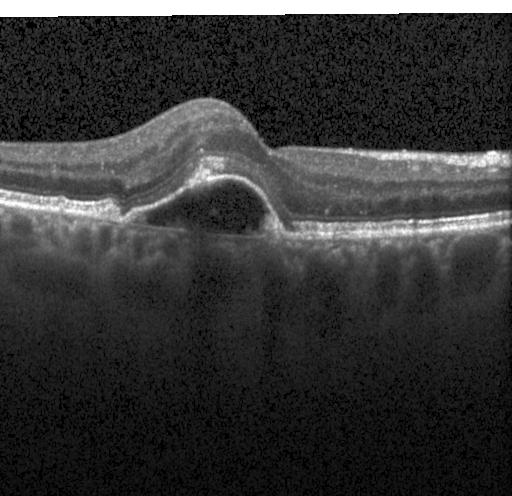 Spectral-domain OCT B-scan: CNV.